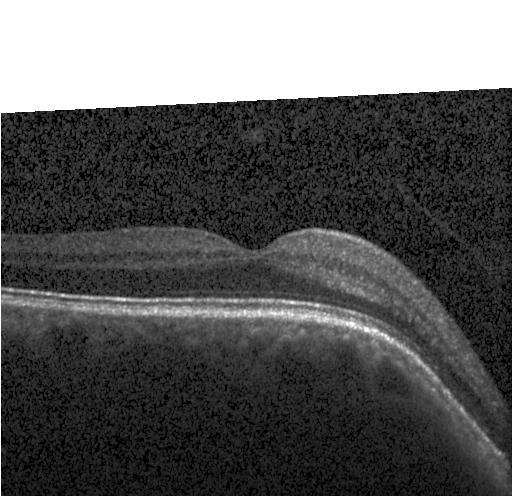
Finding: neither choroidal neovascularization, diabetic macular edema, nor drusen.